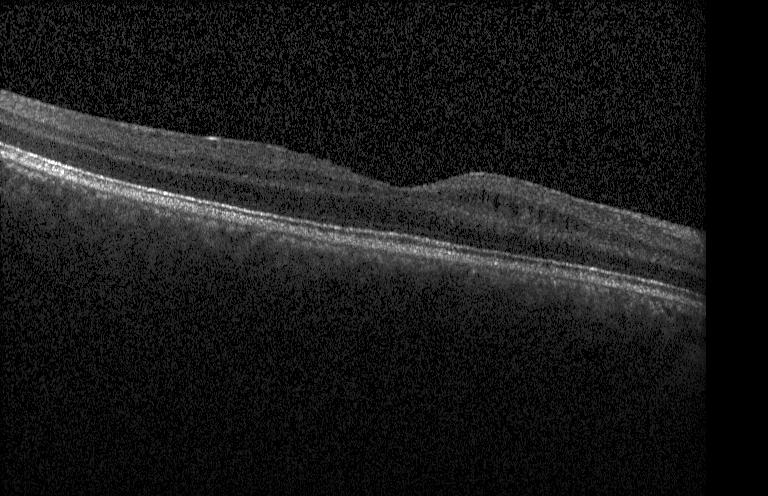

Fovea-centered, retinal OCT B-scan, instrument: Heidelberg Spectralis
Dx: diabetic macular edema (DME).